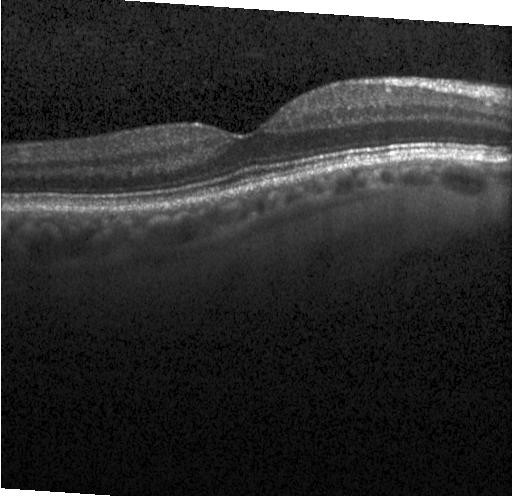 OCT line scan. Heidelberg Spectralis OCT system. Spectral-domain OCT.
Macular OCT: neither choroidal neovascularization, diabetic macular edema, nor drusen.